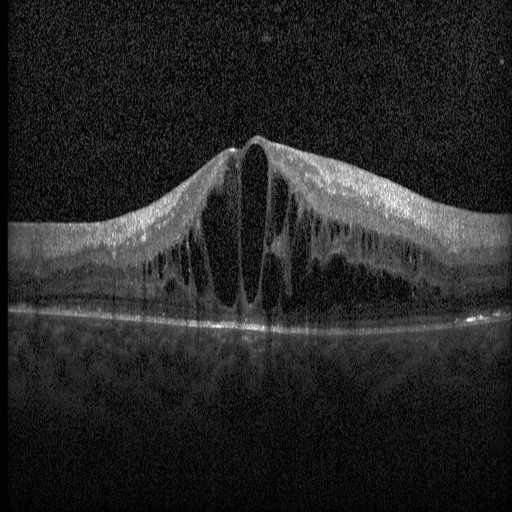 This B-scan demonstrates DME.